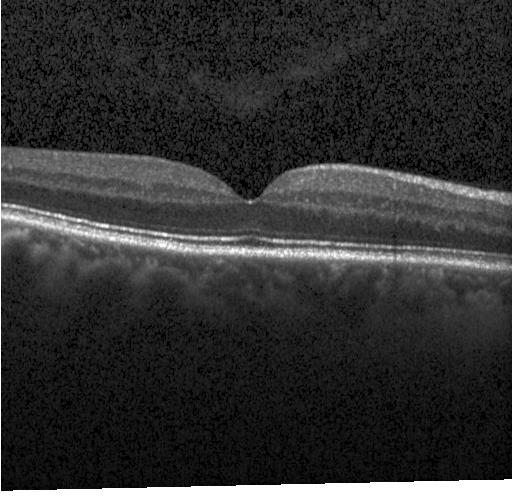
The scan shows neither choroidal neovascularization, diabetic macular edema, nor drusen.